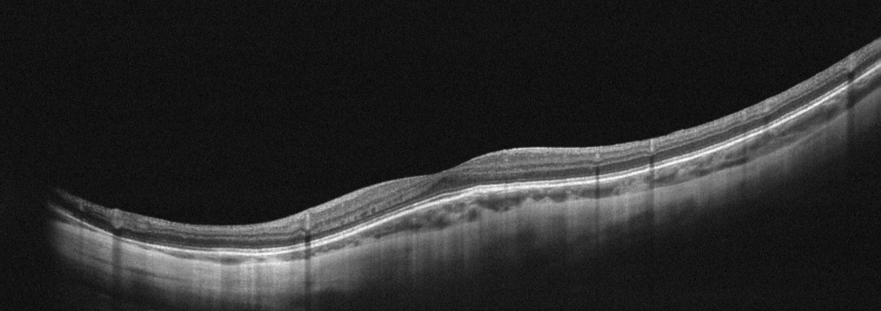
Through the macula; optical coherence tomography B-scan; acquired on an Optovue Avanti RTVue XR
Finding: no evidence of AMD, DME, ERM, RAO, RVO, or VID.